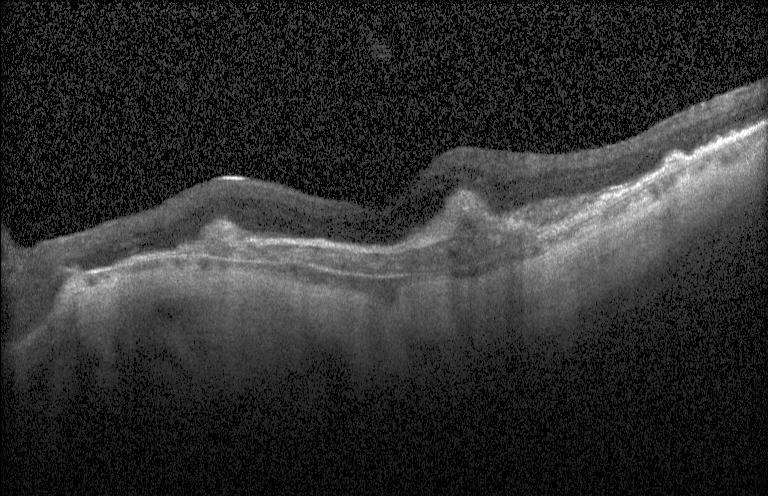
Optical coherence tomography scan — Diagnosis: a choroidal neovascular membrane.